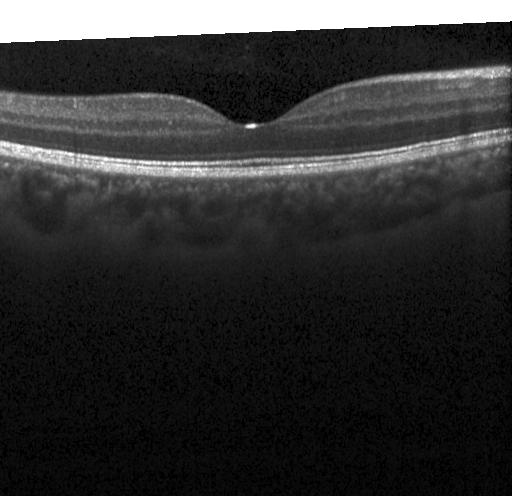

OCT finding: no choroidal neovascularization, no diabetic macular edema, and no drusen.